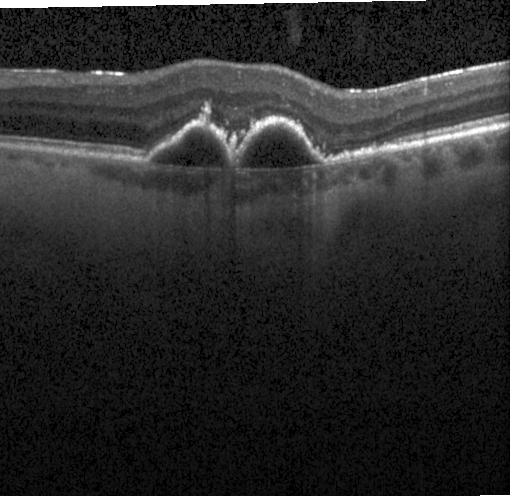

SD-OCT, fovea-centered, optical coherence tomography B-scan, Heidelberg Spectralis OCT system.
This B-scan demonstrates choroidal neovascularization (CNV).